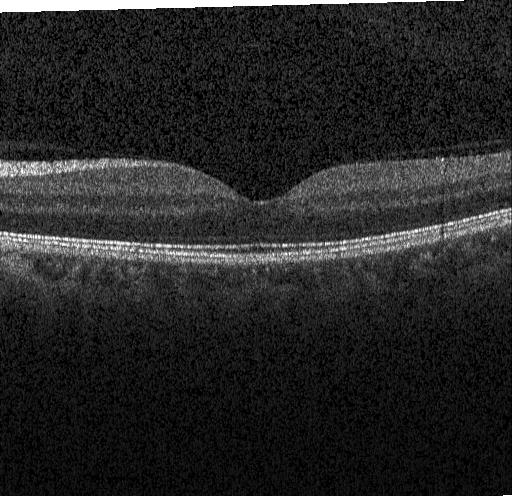

Diagnosis: no evidence of CNV, DME, or drusen.